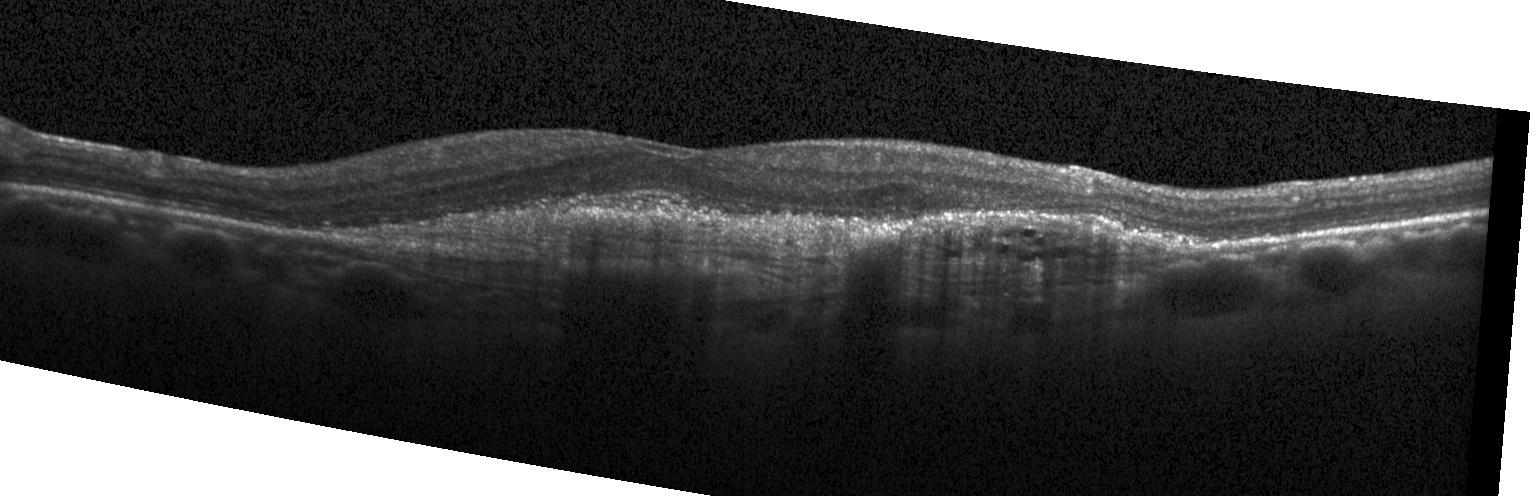 Impression: a choroidal neovascular membrane.